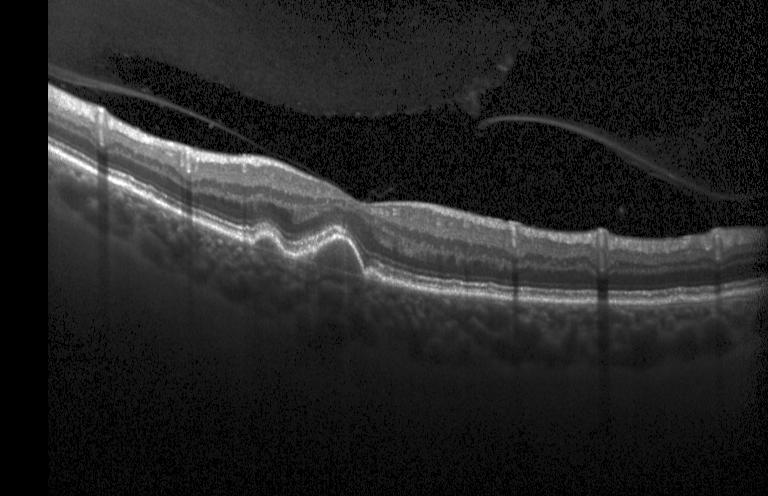 Dx: a choroidal neovascular membrane.